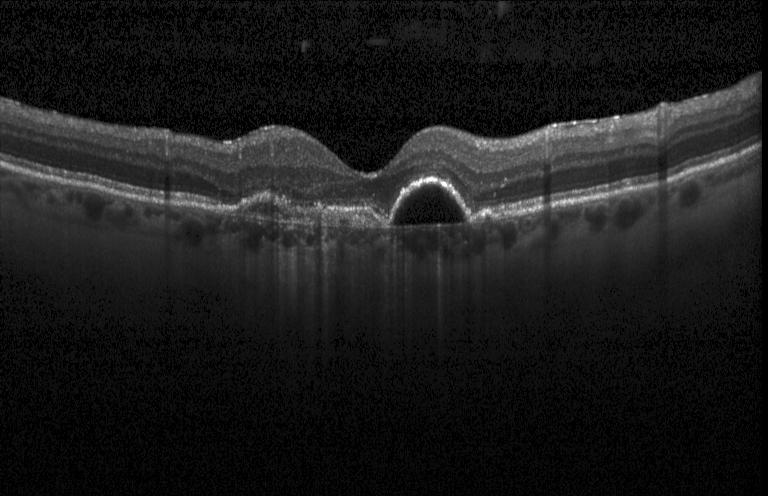
Macular OCT demonstrating choroidal neovascularization (CNV).